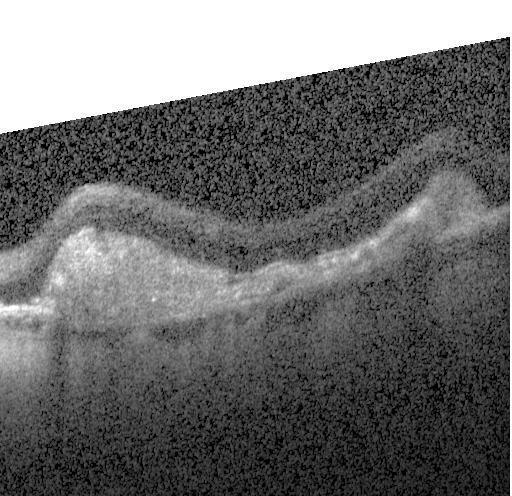
OCT B-scan showing choroidal neovascularization.